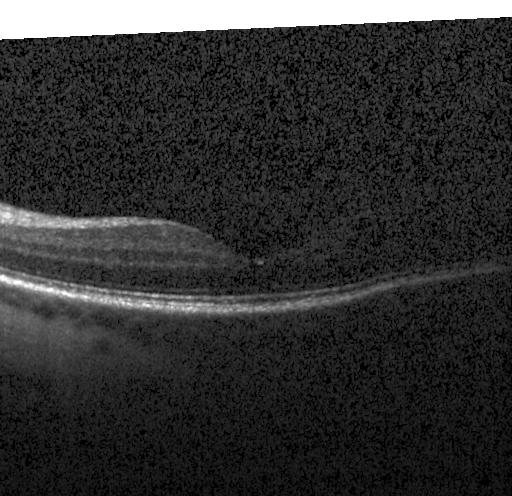

Optical coherence tomography B-scan · centered on the fovea · Heidelberg Spectralis OCT system. Diagnosis: no choroidal neovascularization, diabetic macular edema, or drusen.